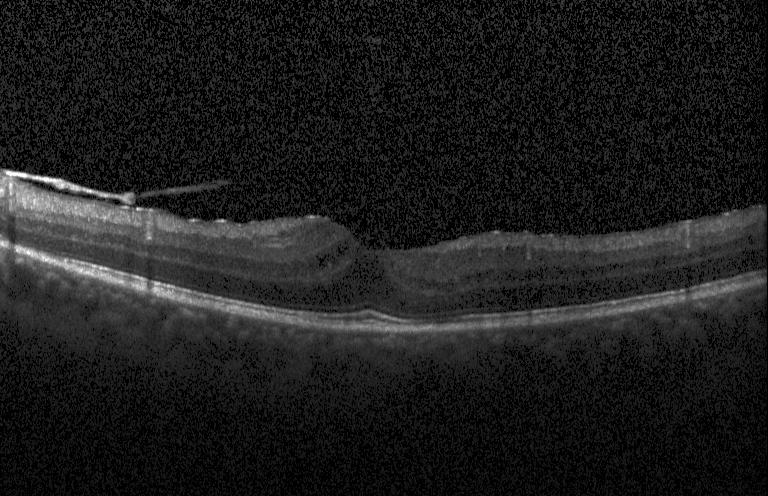 SD-OCT · macular scan · optical coherence tomography scan. Diagnosis: diabetic macular edema.